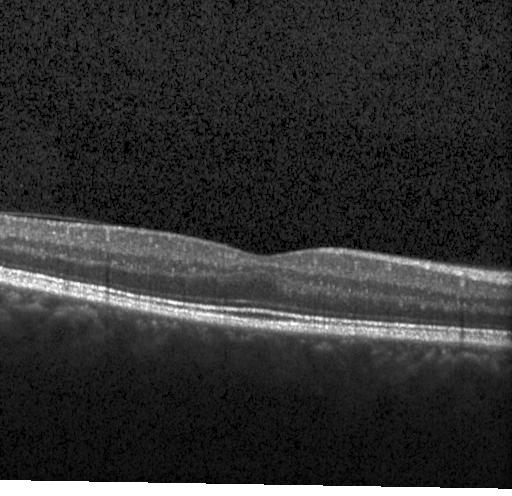 The scan shows no CNV, DME, or drusen.